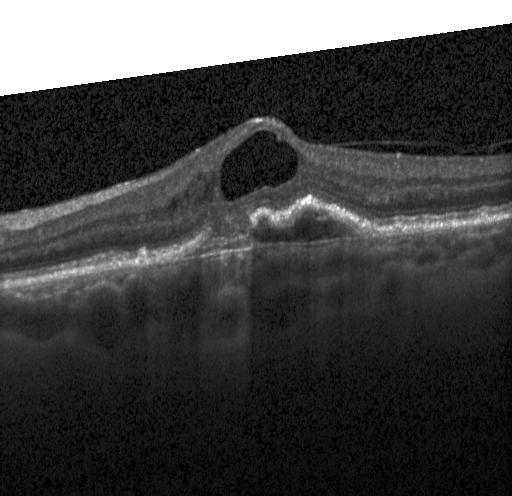

Spectral-domain OCT B-scan: a choroidal neovascular membrane.